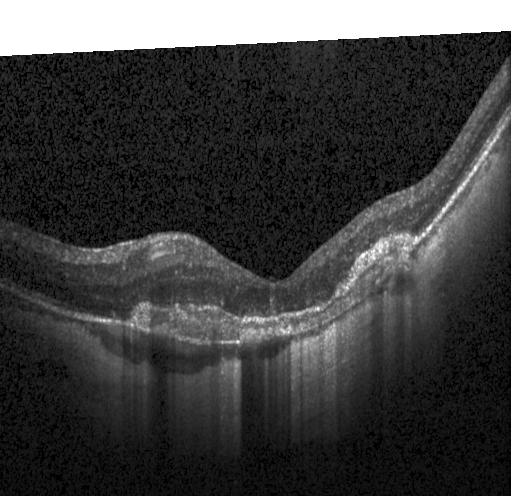

OCT line scan, spectral-domain OCT, macular scan, Heidelberg Spectralis OCT system. Choroidal neovascularization.